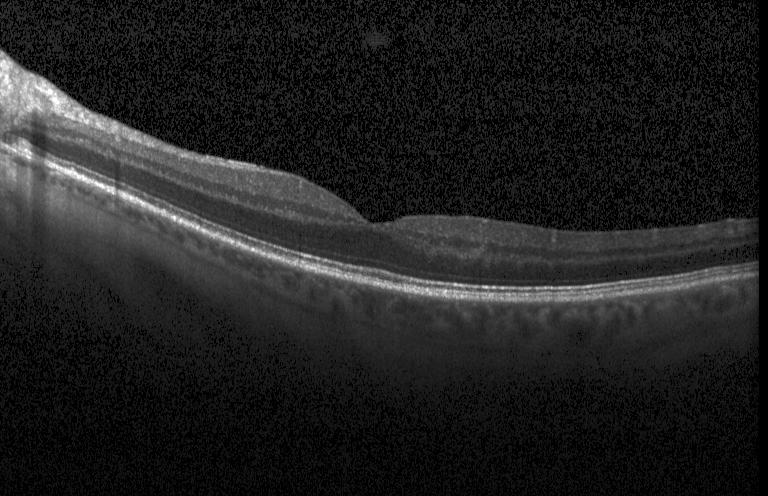
OCT B-scan; acquired on a Heidelberg Spectralis; macular scan. Macular OCT: no choroidal neovascularization, diabetic macular edema, or drusen.